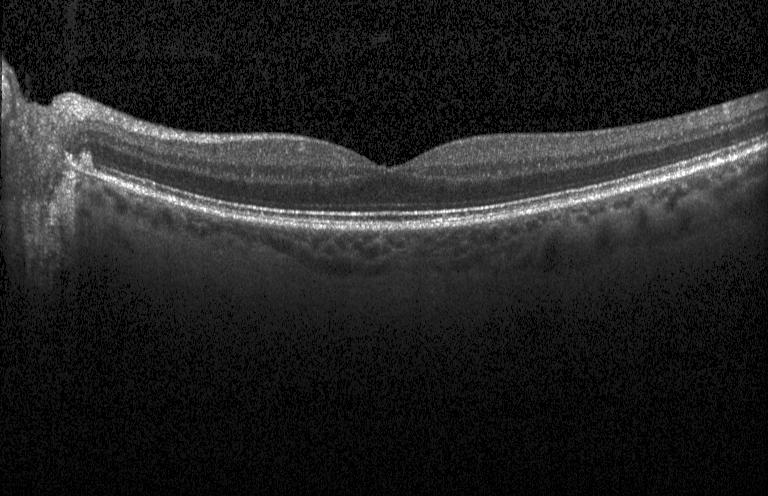

This B-scan demonstrates neither choroidal neovascularization, diabetic macular edema, nor drusen.